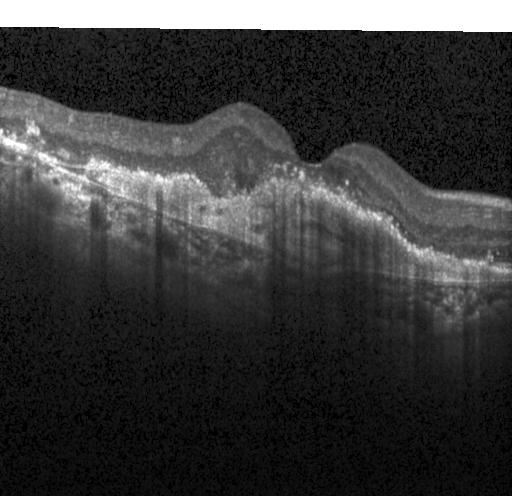 Retinal OCT B-scan.
Impression: a choroidal neovascular membrane.